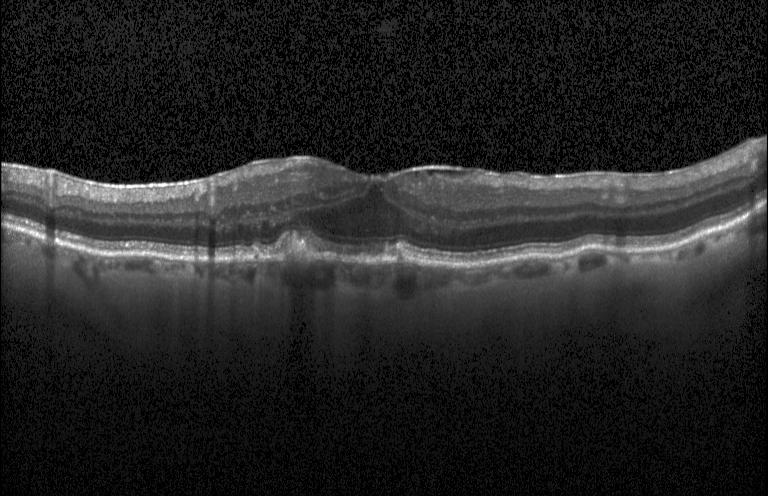 Optical coherence tomography B-scan · SD-OCT · Heidelberg Spectralis · macular scan. Diagnosis: CNV.